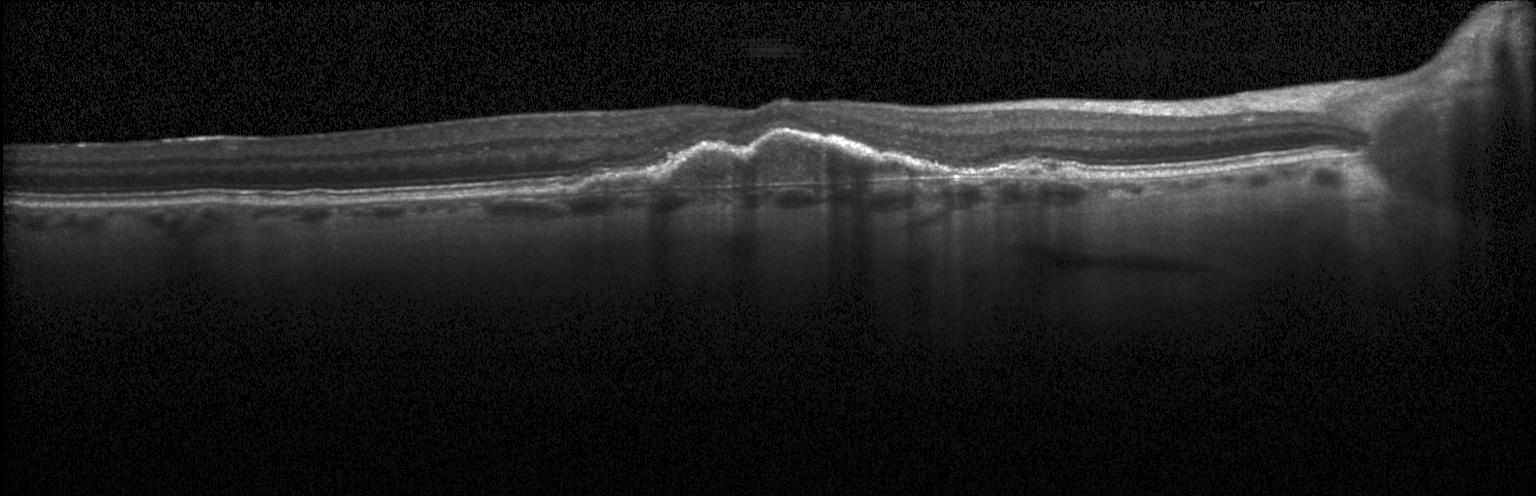

OCT B-scan, instrument: Heidelberg Spectralis, centered on the fovea, SD-OCT. Assessment: choroidal neovascularization (CNV).